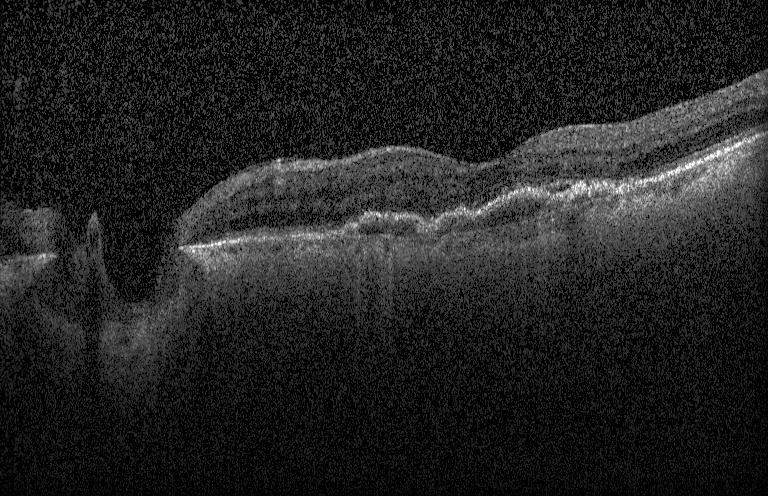

Impression: a choroidal neovascular membrane.